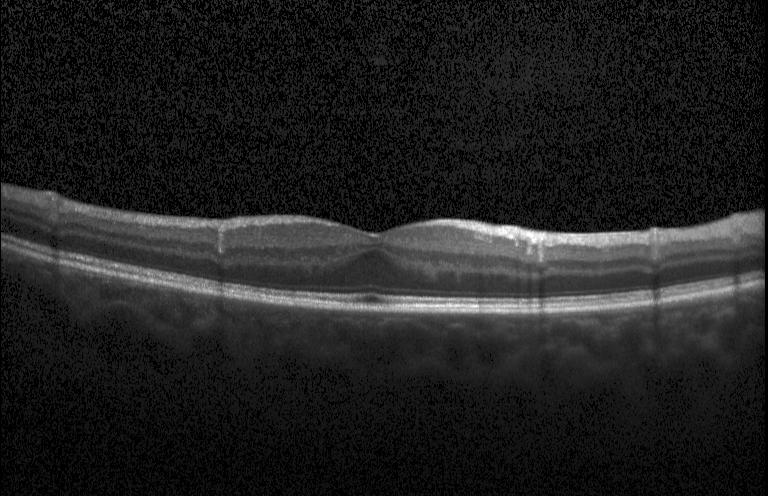 This B-scan demonstrates neither choroidal neovascularization, diabetic macular edema, nor drusen.